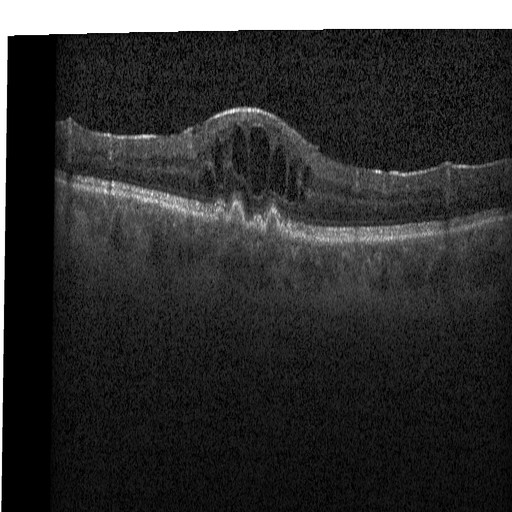 SD-OCT; retinal OCT B-scan; horizontal scan through the fovea; acquired on a Heidelberg Spectralis — Diagnosis: DME.